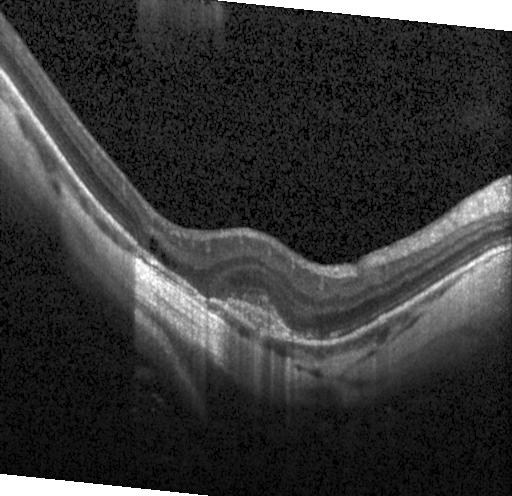
Spectral-domain optical coherence tomography · OCT B-scan. Assessment: a choroidal neovascular membrane.